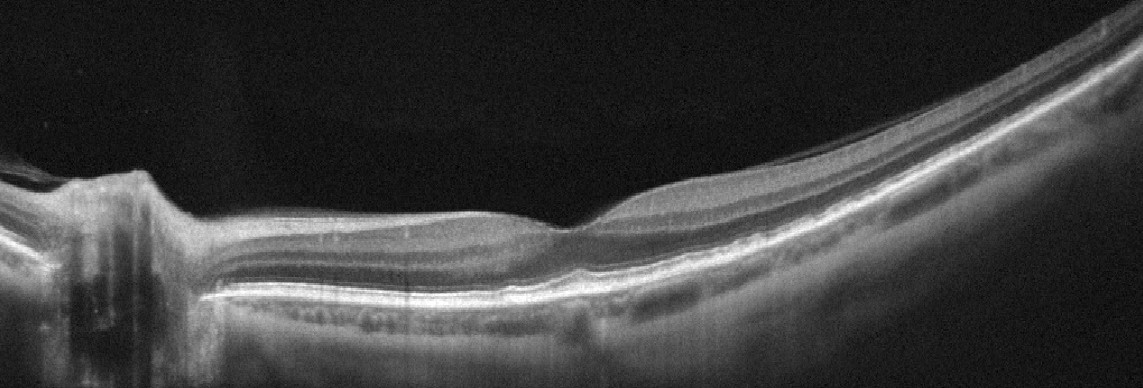

Assessment: age-related macular degeneration (AMD).